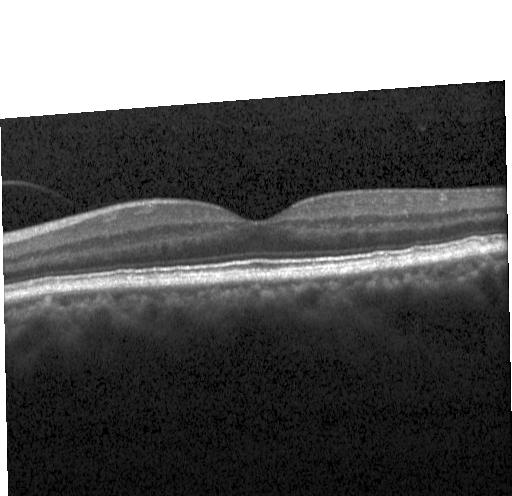
Optical coherence tomography B-scan · SD-OCT · acquired on a Heidelberg Spectralis · macular scan. This B-scan demonstrates no CNV, no DME, and no drusen.